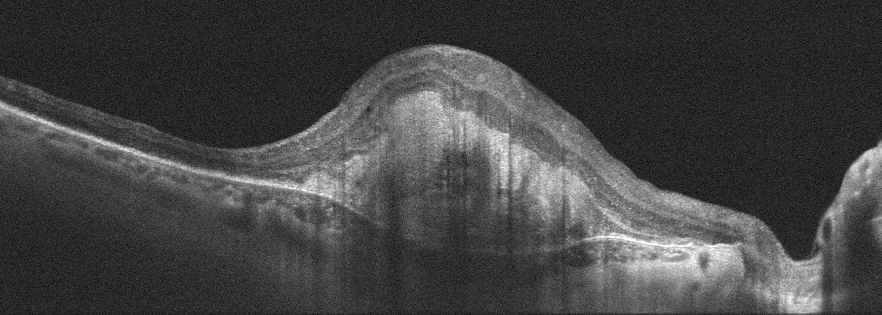
Right eye. OCT line scan — The scan shows AMD.